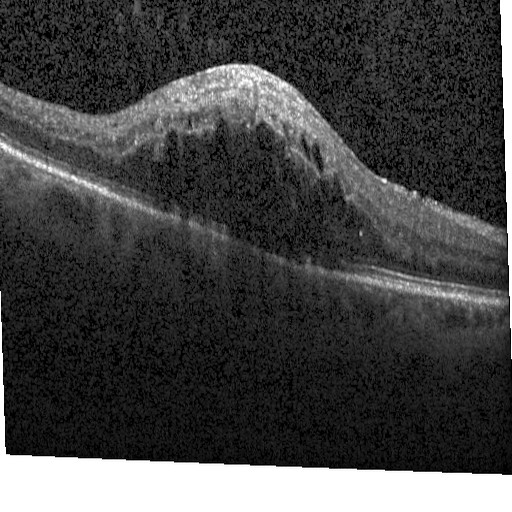

Centered on the fovea. Optical coherence tomography B-scan
Diabetic macular edema (DME).